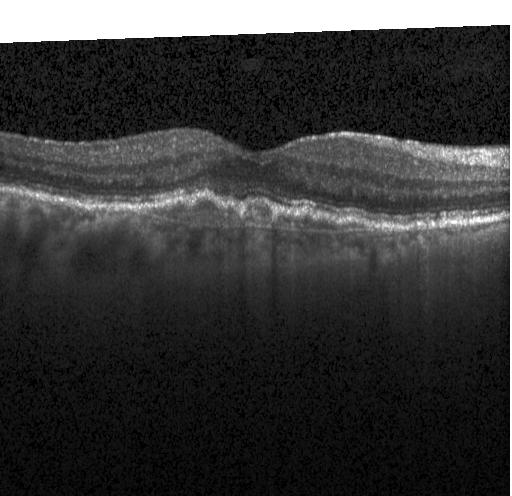

SD-OCT, Heidelberg Spectralis, OCT line scan. Dx: a choroidal neovascular membrane.